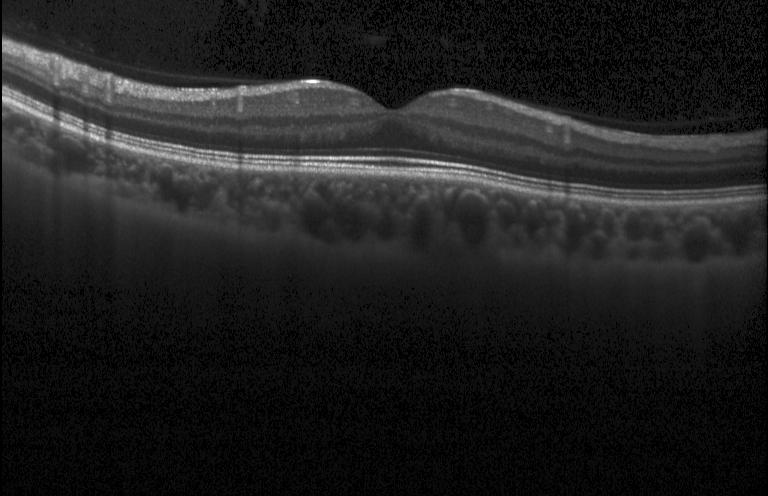
Macular scan, spectral-domain OCT, instrument: Heidelberg Spectralis, OCT B-scan — Impression: no CNV, no DME, and no drusen.